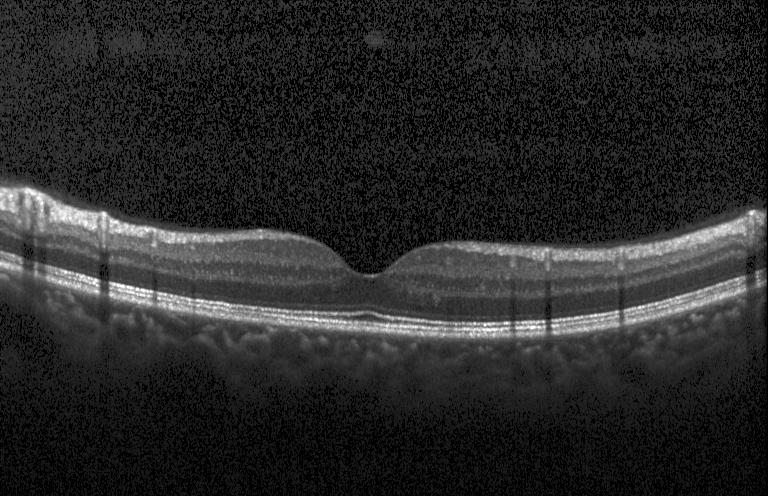

Spectral-domain optical coherence tomography; retinal OCT B-scan; through the macula; instrument: Heidelberg Spectralis. Impression: neither choroidal neovascularization, diabetic macular edema, nor drusen.